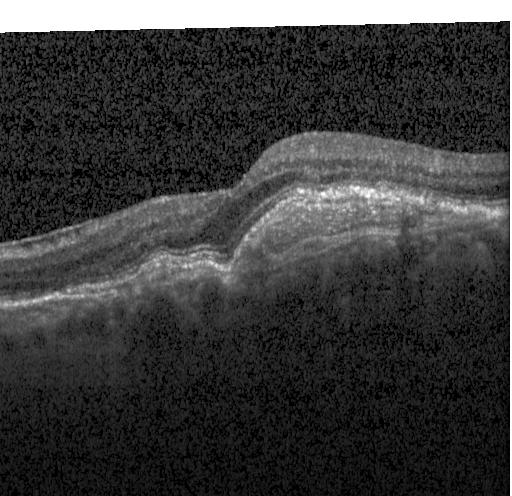 Choroidal neovascularization (CNV).